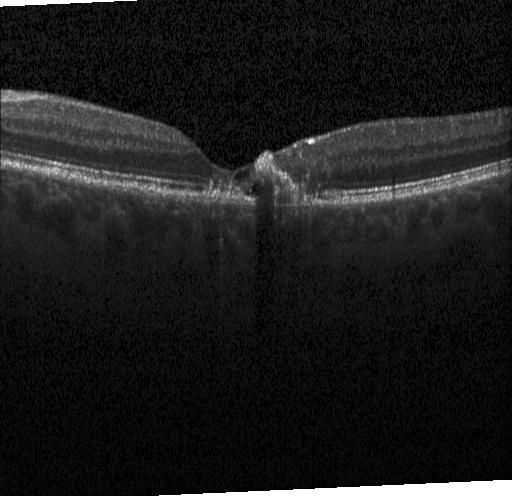
Optical coherence tomography B-scan, spectral-domain optical coherence tomography, Heidelberg Spectralis, fovea-centered. Assessment: CNV.